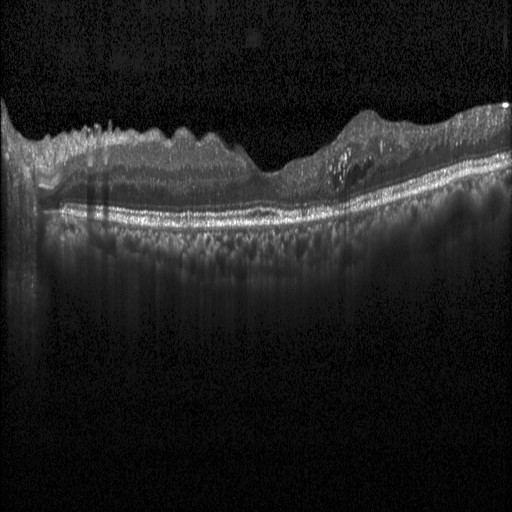

Acquired on a Heidelberg Spectralis, optical coherence tomography scan, centered on the fovea
The scan shows diabetic macular edema.